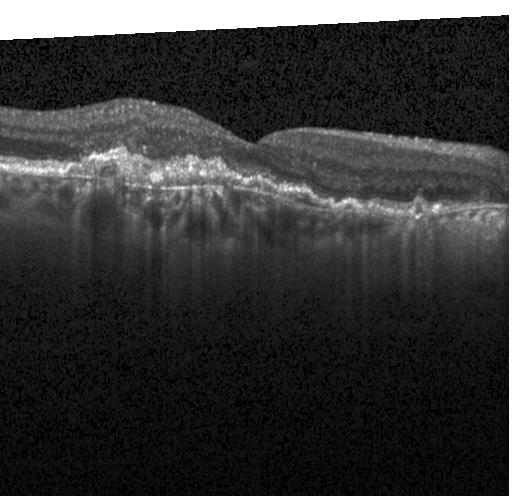

OCT B-scan — Finding: a choroidal neovascular membrane.